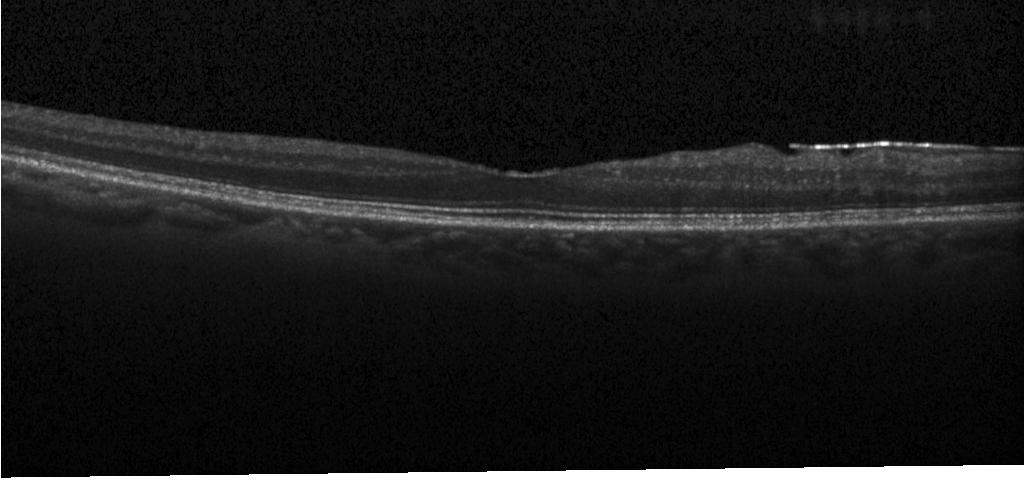 No choroidal neovascularization, diabetic macular edema, or drusen.